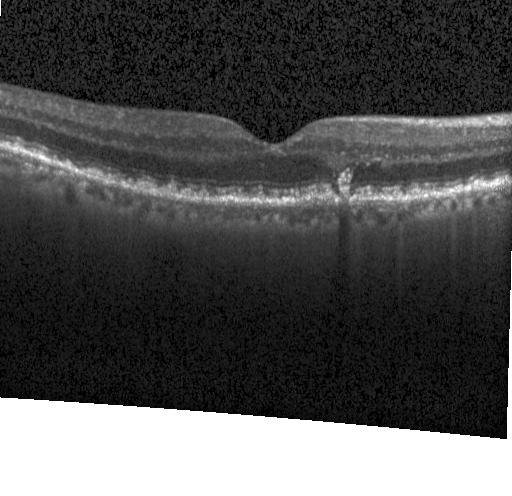
Impression: drusen.